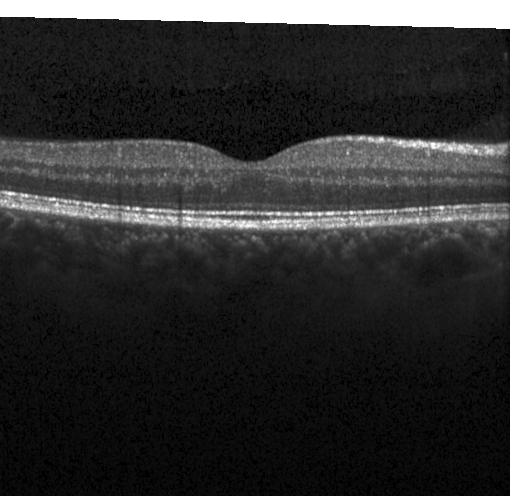
Finding: no choroidal neovascularization, diabetic macular edema, or drusen.